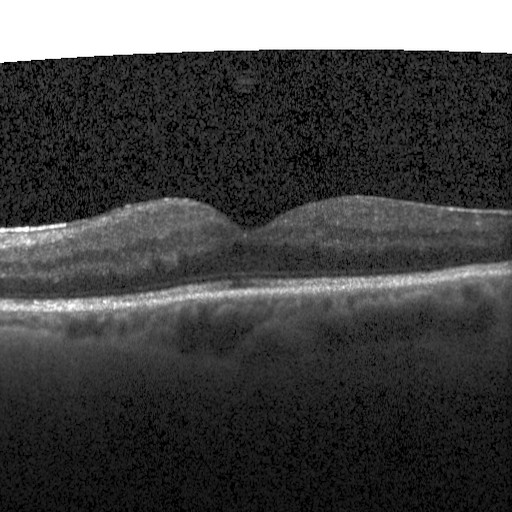

Impression: diabetic macular edema.